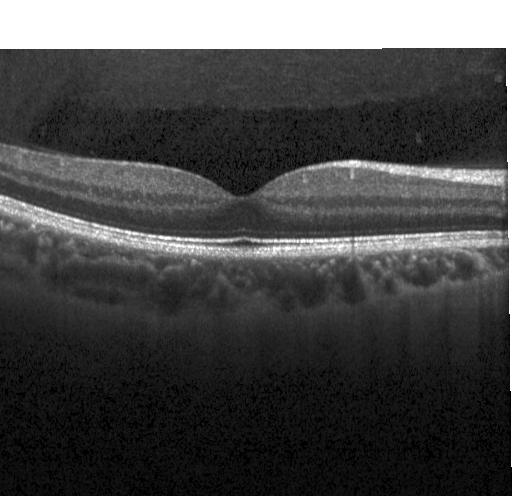

Retinal OCT B-scan. Through the macula. Impression: no choroidal neovascularization, no diabetic macular edema, and no drusen.